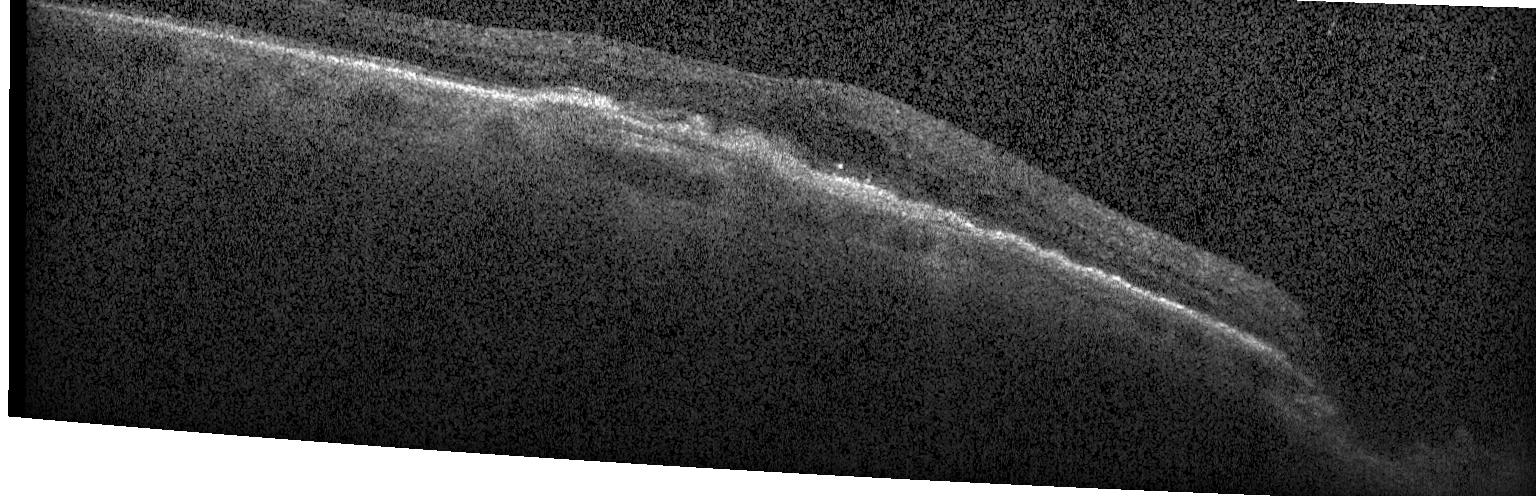

Retinal OCT B-scan · SD-OCT — Dx: a choroidal neovascular membrane.